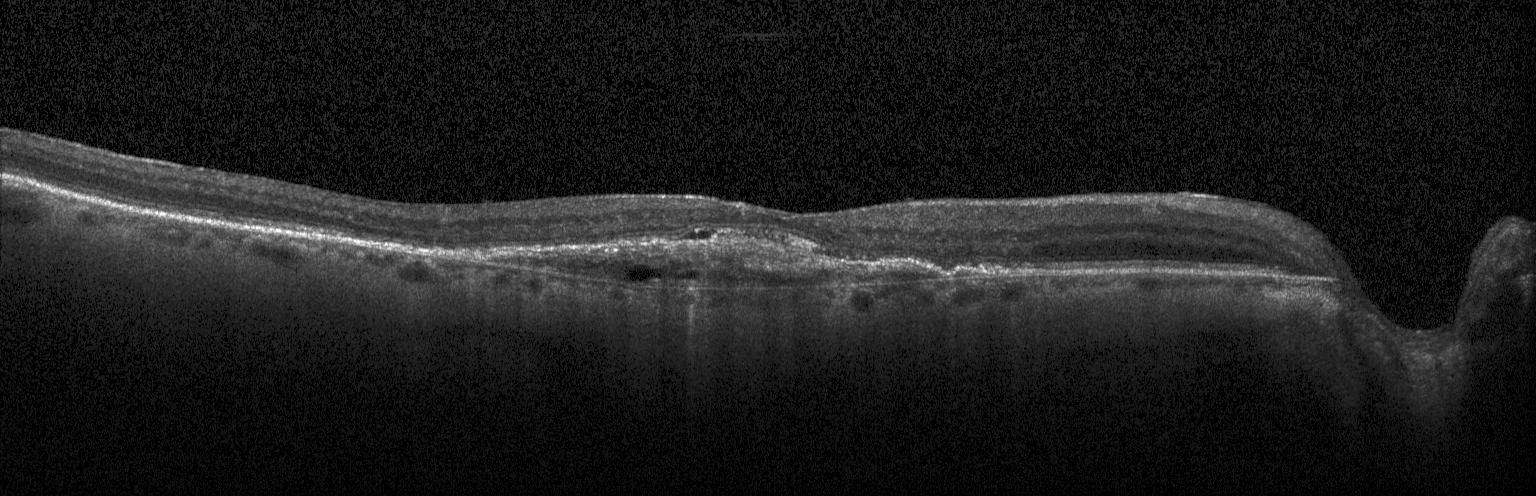

OCT line scan
A choroidal neovascular membrane.